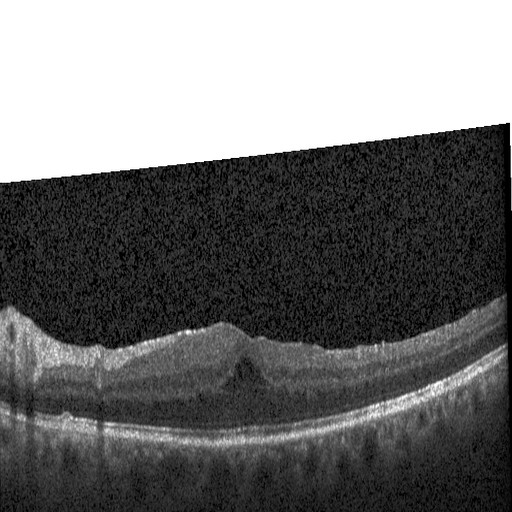 Fovea-centered. Heidelberg Spectralis. Optical coherence tomography scan. Spectral-domain optical coherence tomography. Finding: diabetic macular edema.